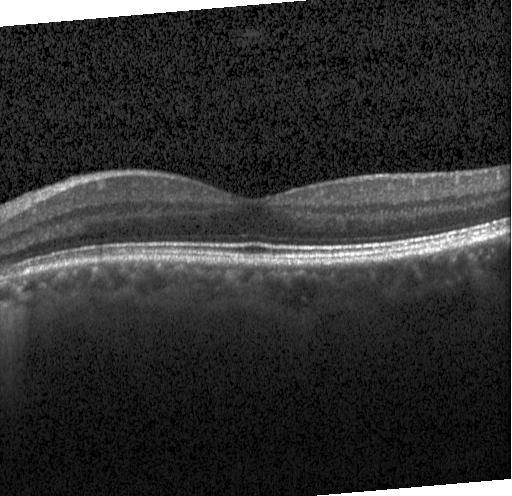 The scan shows neither choroidal neovascularization, diabetic macular edema, nor drusen.